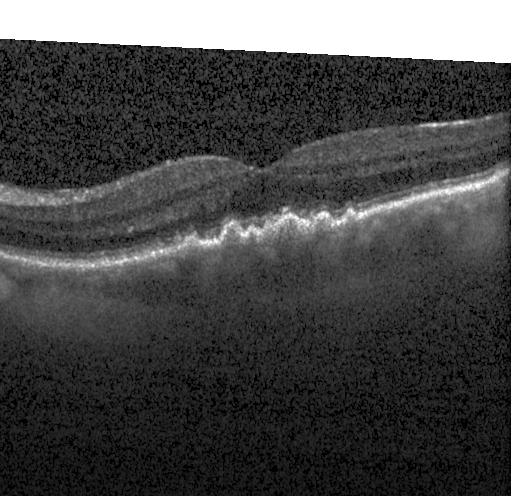 Diagnosis: sub-RPE drusenoid deposits.